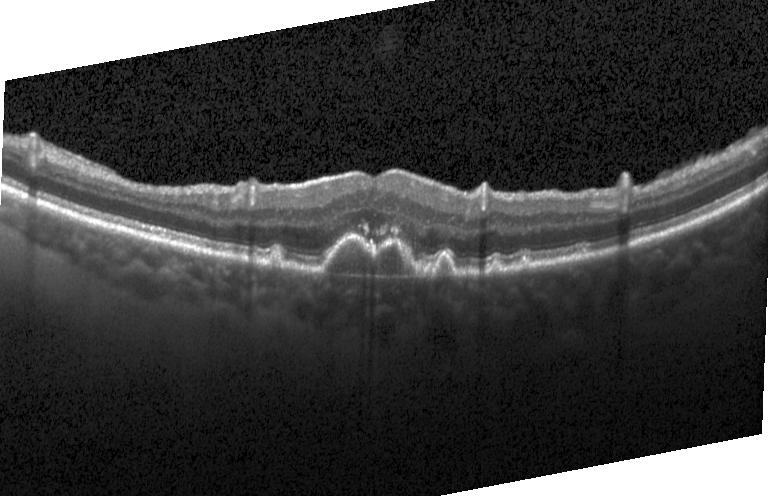 Instrument: Heidelberg Spectralis · spectral-domain optical coherence tomography · centered on the fovea · retinal OCT B-scan. Impression: multiple drusen.